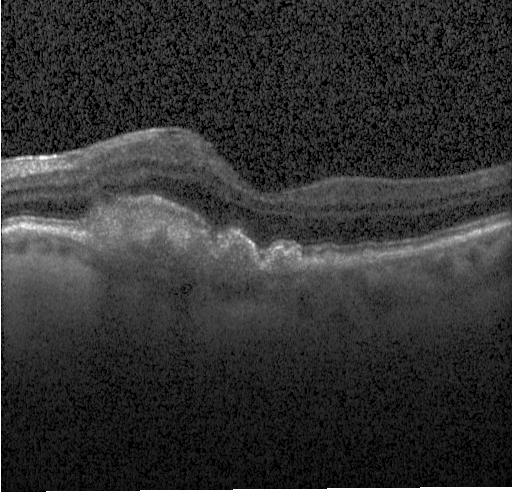 Optical coherence tomography B-scan · acquired on a Heidelberg Spectralis · spectral-domain optical coherence tomography.
Impression: choroidal neovascularization (CNV).